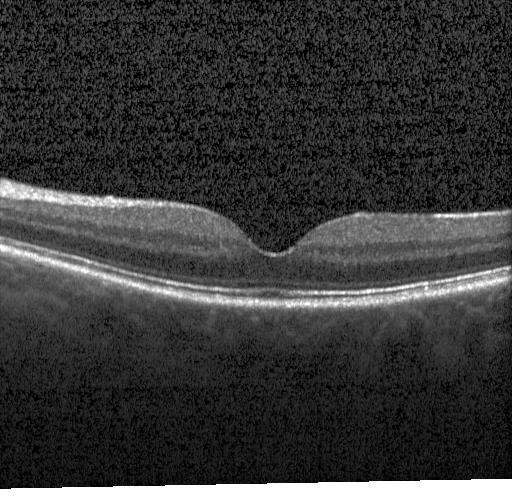 No choroidal neovascularization, diabetic macular edema, or drusen.